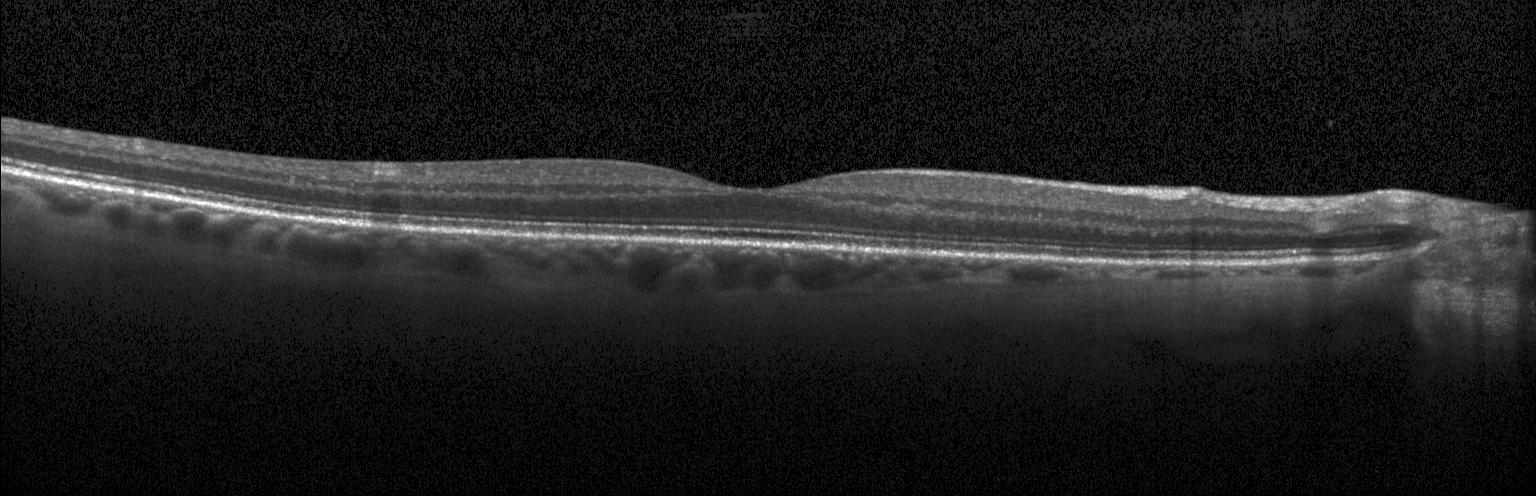
Horizontal scan through the fovea · instrument: Heidelberg Spectralis · OCT B-scan · SD-OCT — No choroidal neovascularization, diabetic macular edema, or drusen.